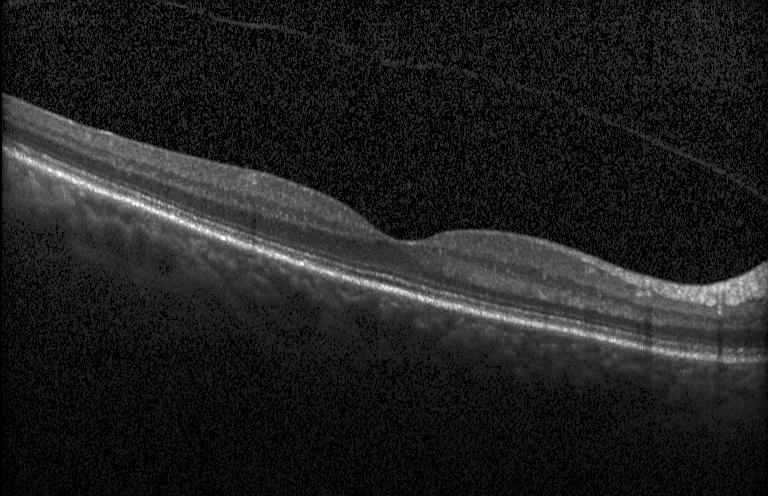
The scan shows no evidence of choroidal neovascularization, diabetic macular edema, or drusen.